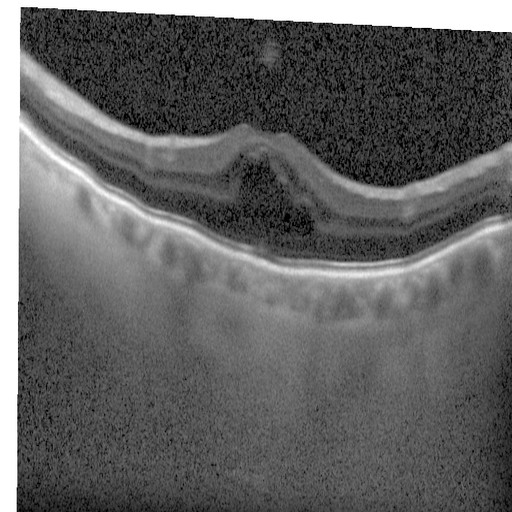
Acquired on a Heidelberg Spectralis, optical coherence tomography B-scan.
Assessment: diabetic macular edema.